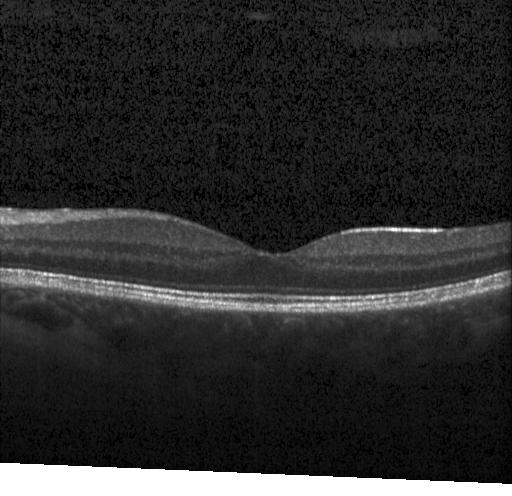 Retinal OCT B-scan · Heidelberg Spectralis OCT system · horizontal scan through the fovea.
No evidence of CNV, DME, or drusen.